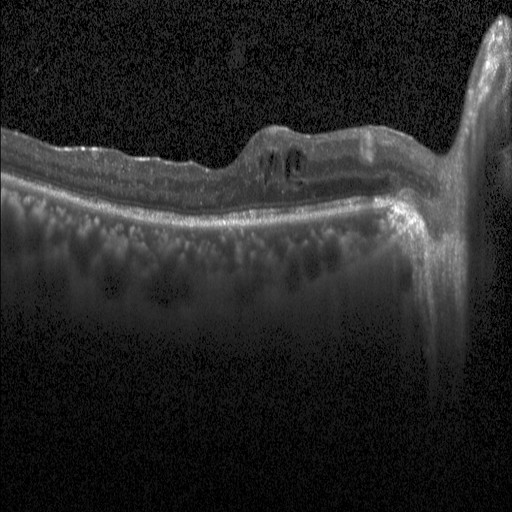 Retinal OCT B-scan.
Diagnosis: diabetic macular edema (DME).